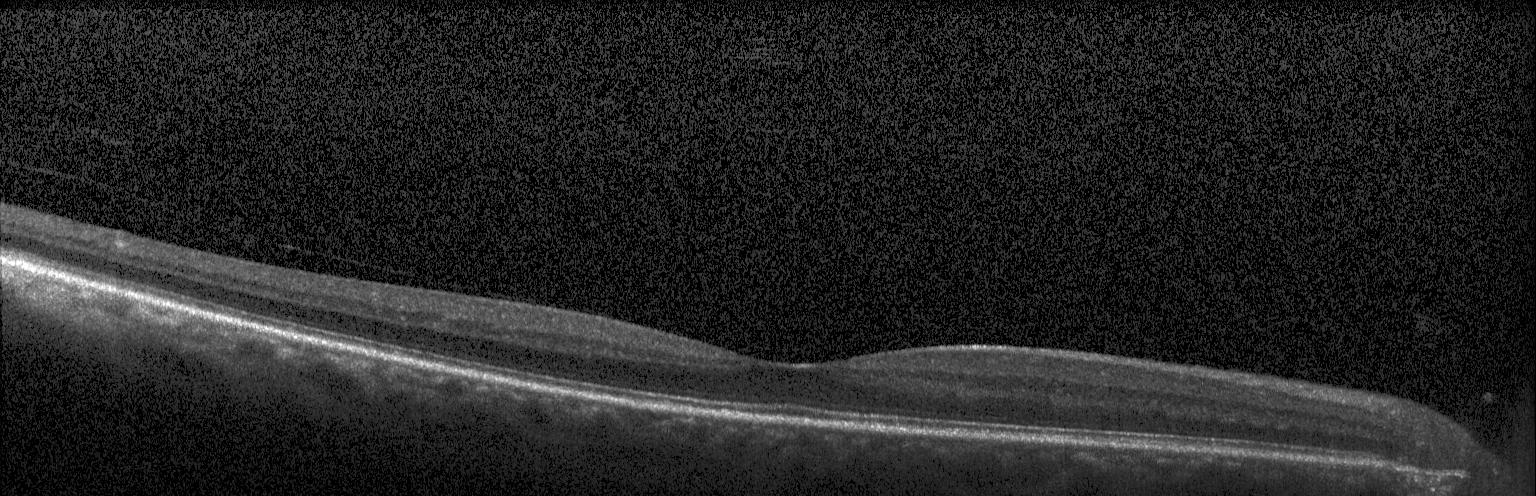

Heidelberg Spectralis OCT system · retinal OCT cross-section · SD-OCT. Impression: no CNV, no DME, and no drusen.